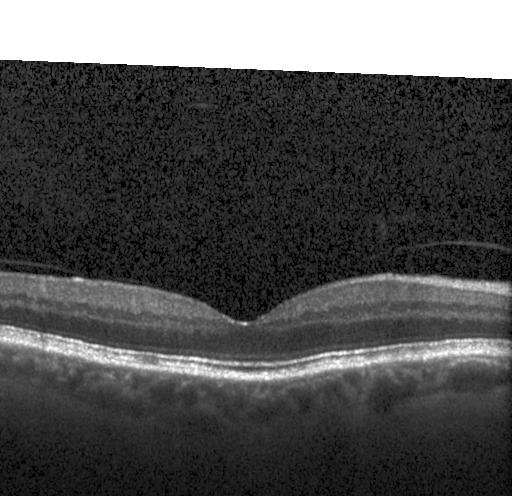

Acquired on a Heidelberg Spectralis; through the macula; retinal OCT cross-section. Impression: no choroidal neovascularization, diabetic macular edema, or drusen.